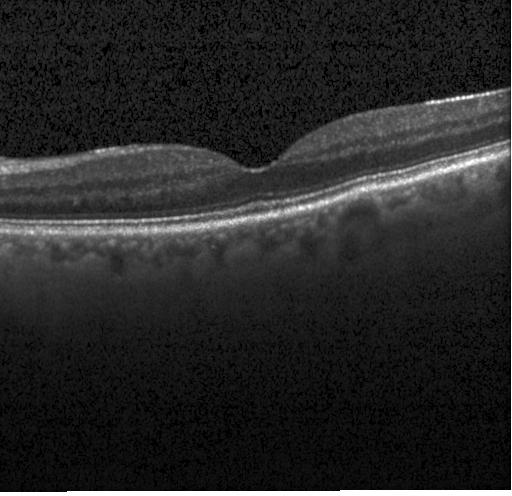
Impression: neither choroidal neovascularization, diabetic macular edema, nor drusen.